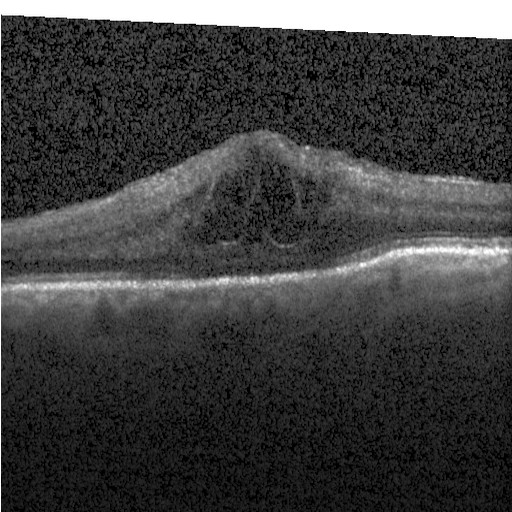 Fovea-centered · optical coherence tomography B-scan.
Impression: diabetic macular edema (DME).